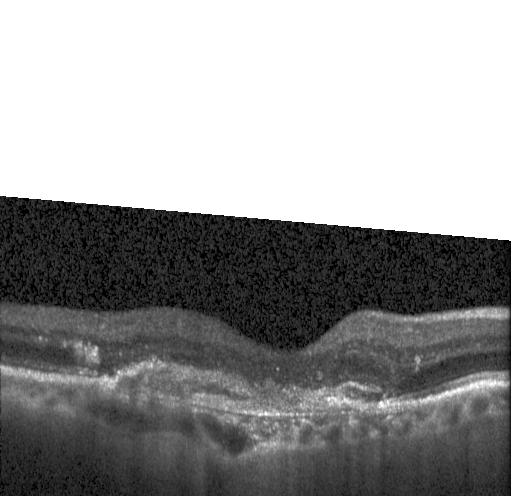

OCT scan showing a choroidal neovascular membrane.